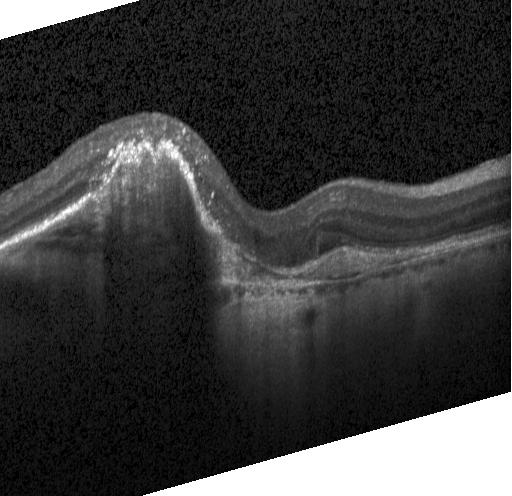

Diagnosis: CNV.